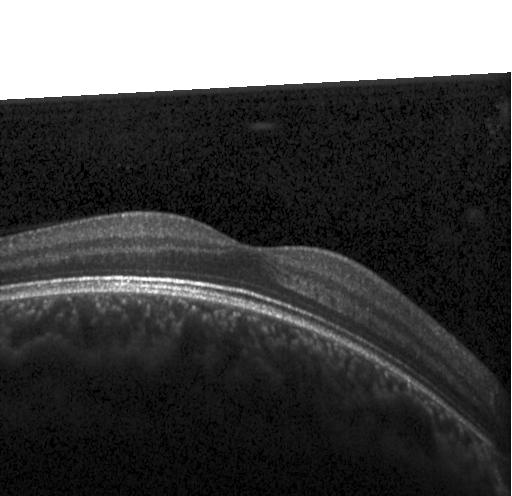
Retinal OCT cross-section showing no choroidal neovascularization, diabetic macular edema, or drusen.